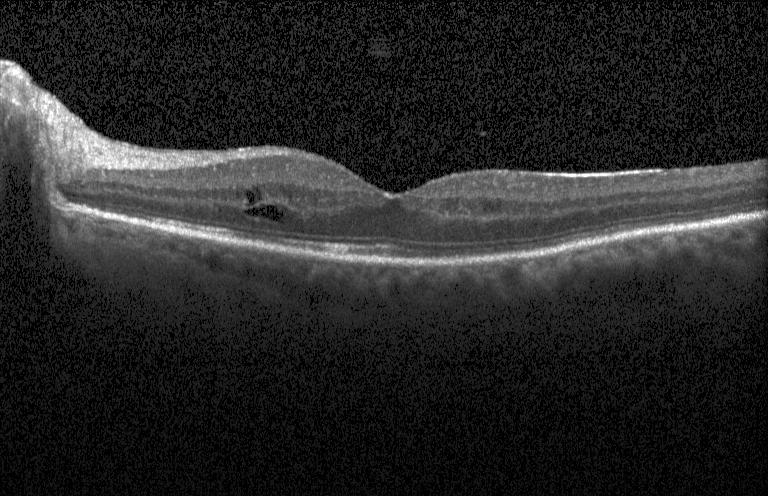 Retinal OCT cross-section — Macular OCT: diabetic macular edema (DME).